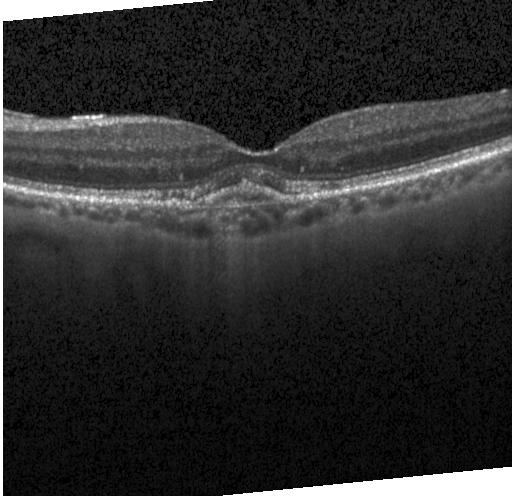
Retinal OCT cross-section · SD-OCT — Macular OCT: a choroidal neovascular membrane.